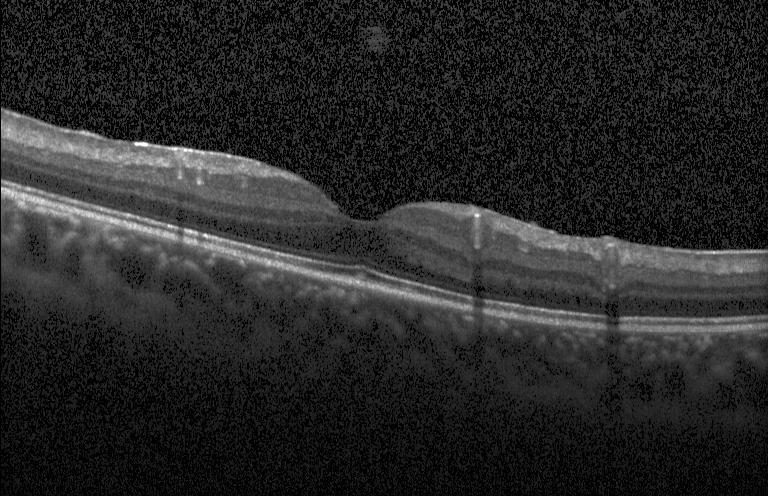
Impression: no CNV, no DME, and no drusen.